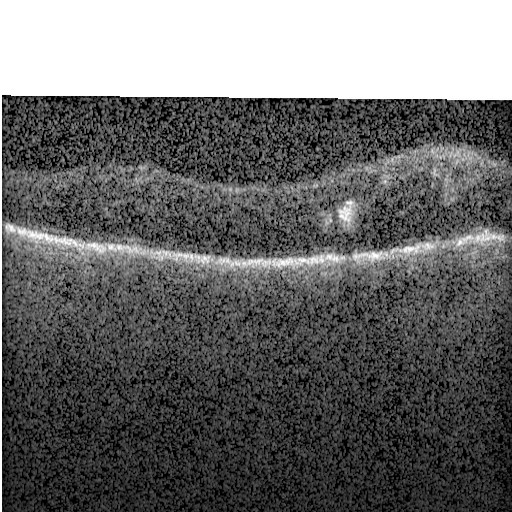

OCT B-scan; instrument: Heidelberg Spectralis — Assessment: diabetic macular edema (DME).